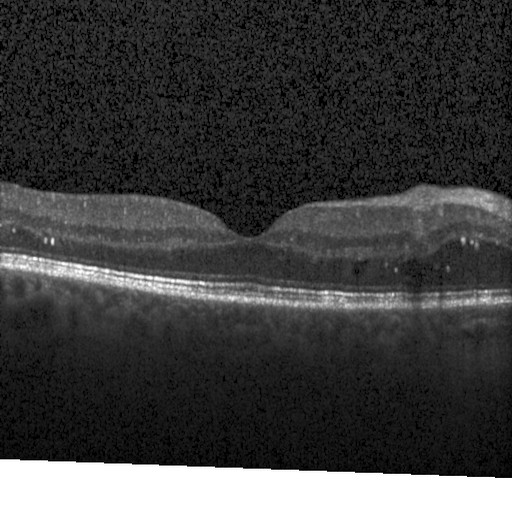
SD-OCT. OCT line scan. Centered on the fovea.
Dx: diabetic macular edema (DME).